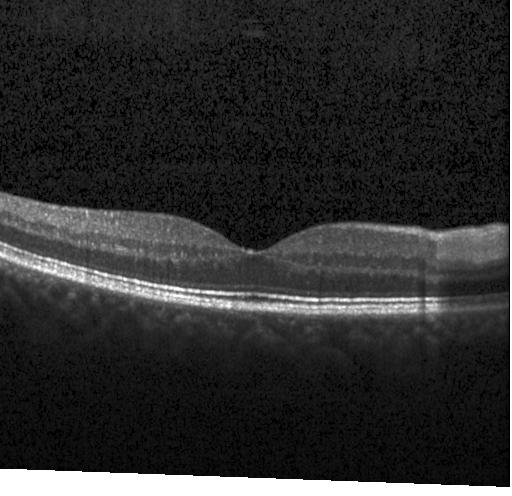

SD-OCT; optical coherence tomography B-scan
The scan shows no choroidal neovascularization, no diabetic macular edema, and no drusen.